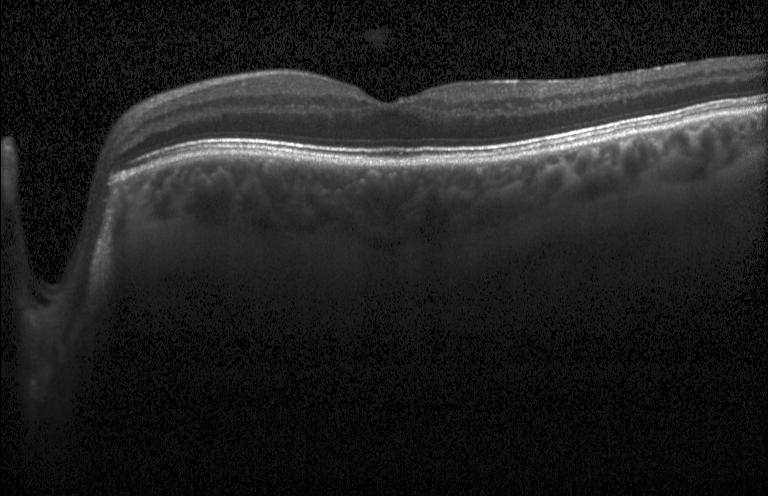
Optical coherence tomography scan · through the macula · spectral-domain optical coherence tomography · instrument: Heidelberg Spectralis
OCT finding: no evidence of choroidal neovascularization, diabetic macular edema, or drusen.